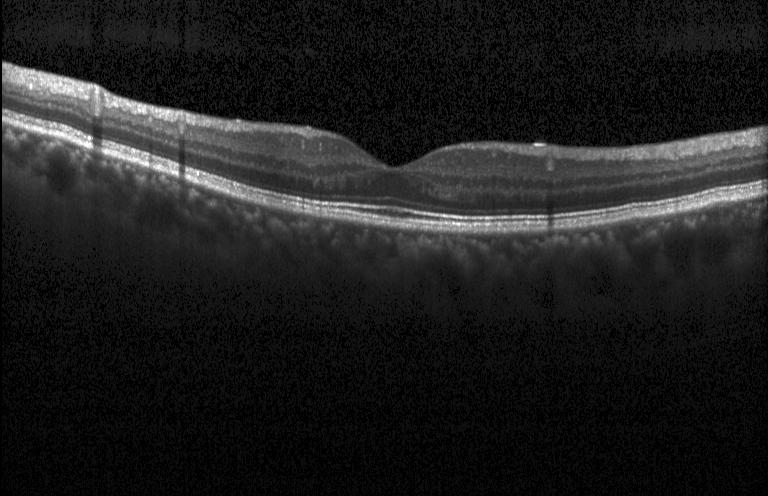 Macular OCT demonstrating no evidence of CNV, DME, or drusen.